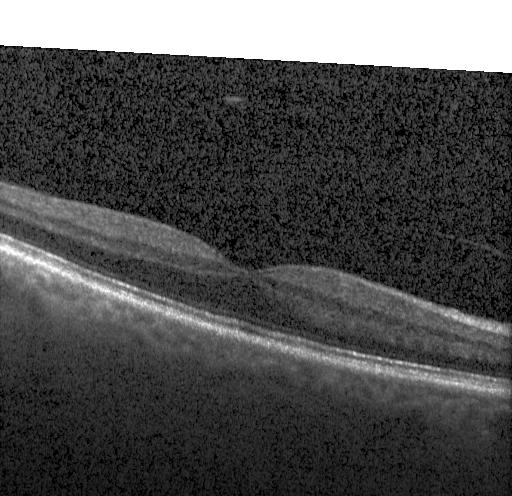

OCT scan showing no evidence of CNV, DME, or drusen.